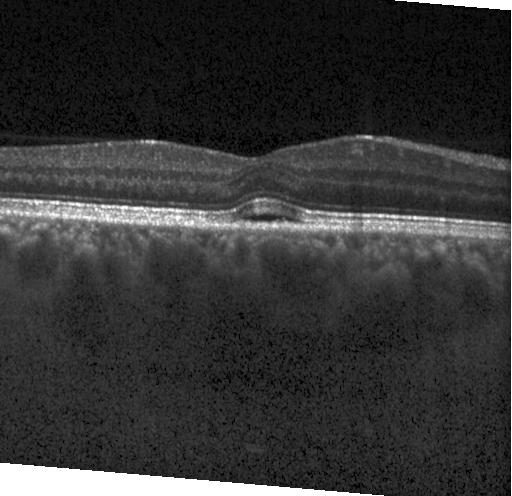

OCT B-scan showing CNV.